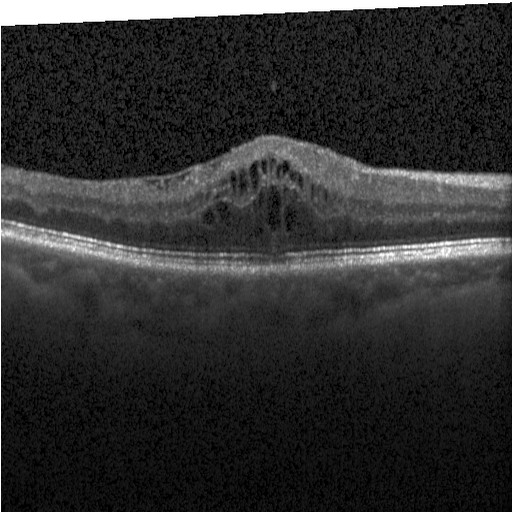 Optical coherence tomography B-scan. The scan shows DME.